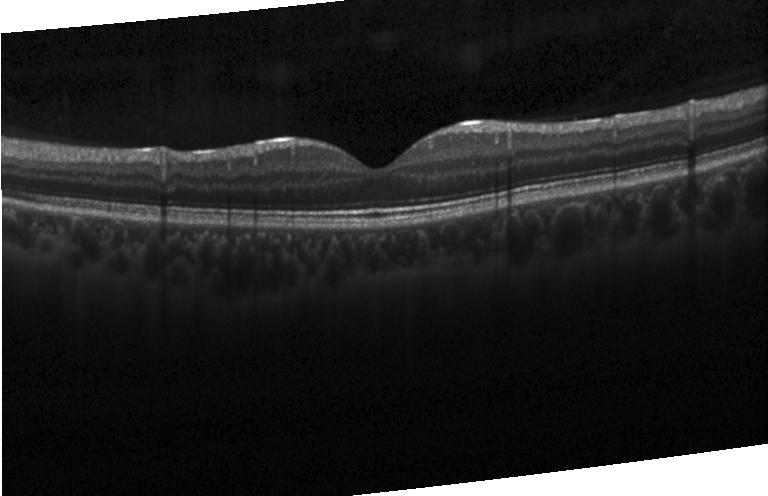 OCT line scan
Assessment: no evidence of CNV, DME, or drusen.